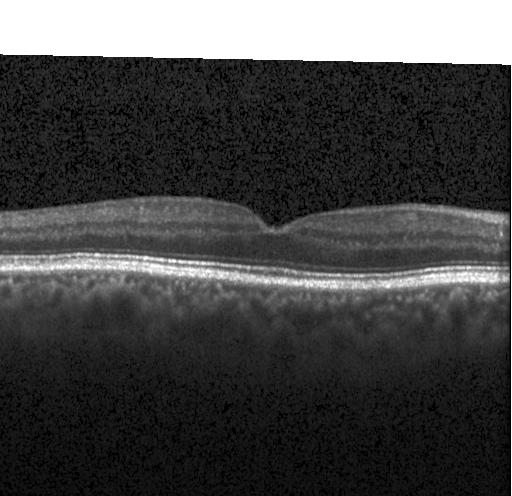
Macular OCT: no CNV, no DME, and no drusen.